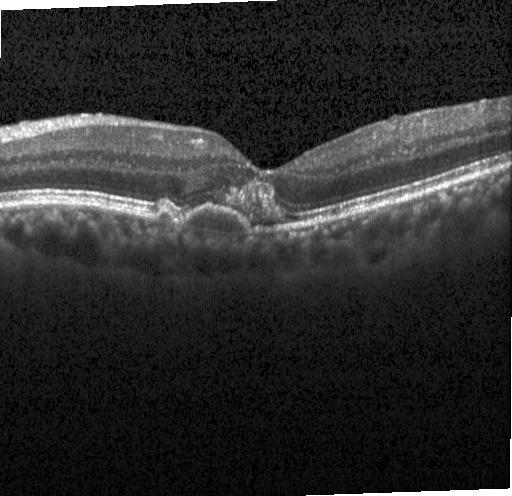
Diagnosis: a choroidal neovascular membrane.